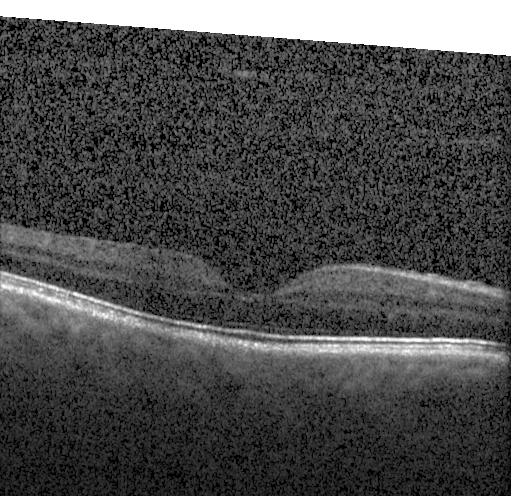

Retinal OCT cross-section — Diagnosis: no evidence of choroidal neovascularization, diabetic macular edema, or drusen.